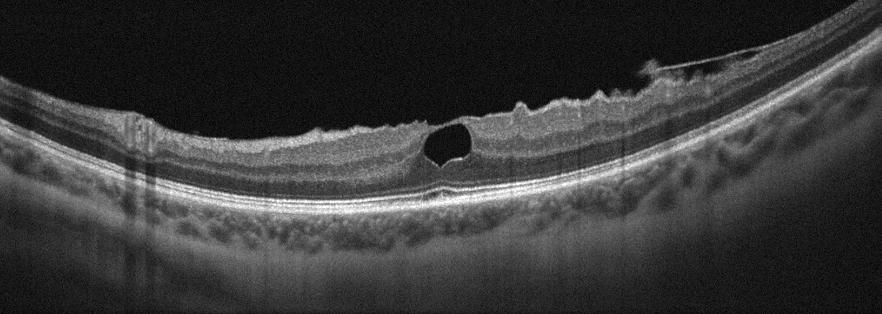

Optical coherence tomography B-scan, instrument: Optovue Avanti RTVue XR, OS, fovea-centered.
Diagnosis: ERM.